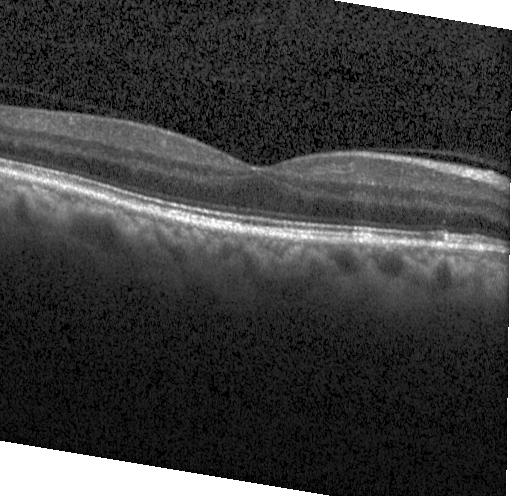 Acquired on a Heidelberg Spectralis · retinal OCT cross-section · spectral-domain OCT.
No evidence of CNV, DME, or drusen.